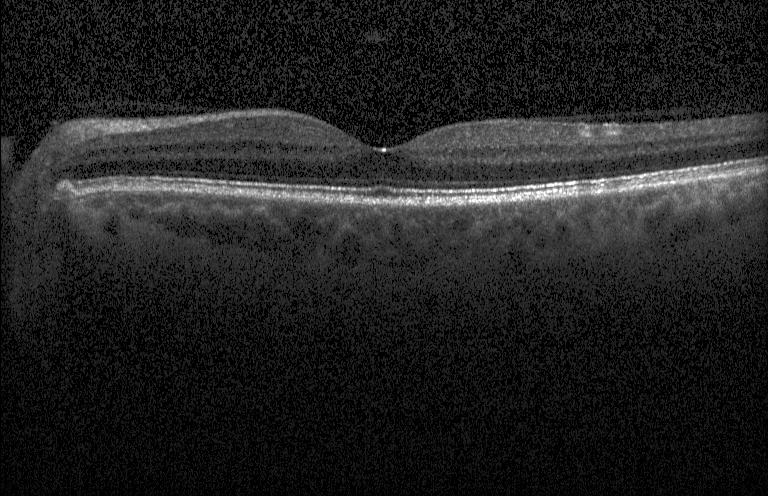
This B-scan demonstrates no evidence of choroidal neovascularization, diabetic macular edema, or drusen.